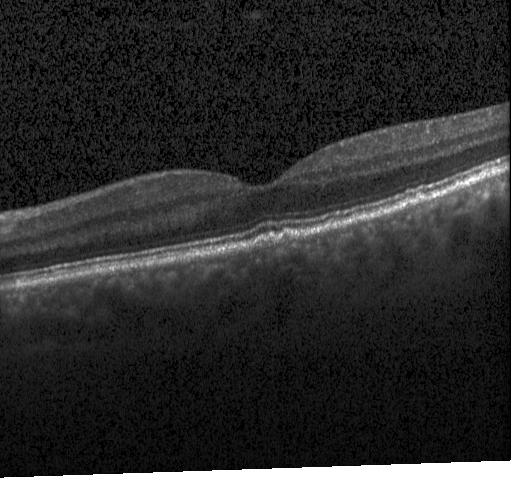 OCT B-scan
Diagnosis: sub-RPE drusenoid deposits.